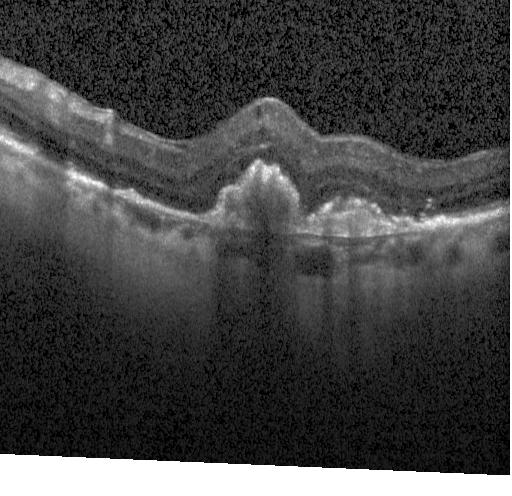 OCT line scan
This B-scan demonstrates a choroidal neovascular membrane.